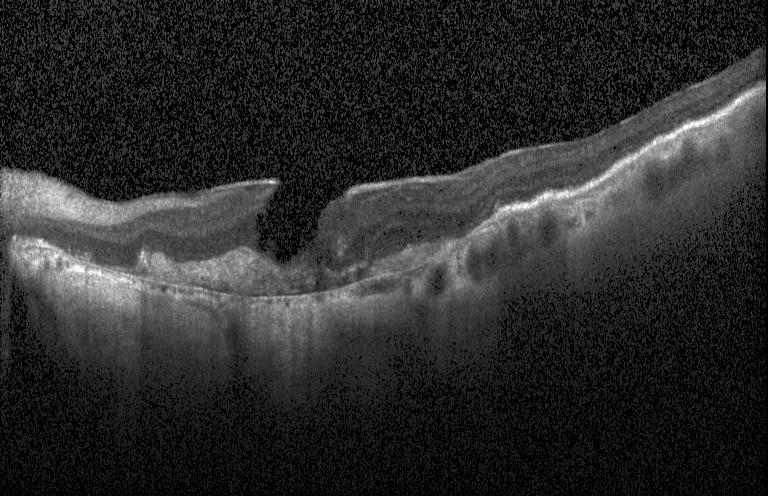
Optical coherence tomography scan — The scan shows a choroidal neovascular membrane.